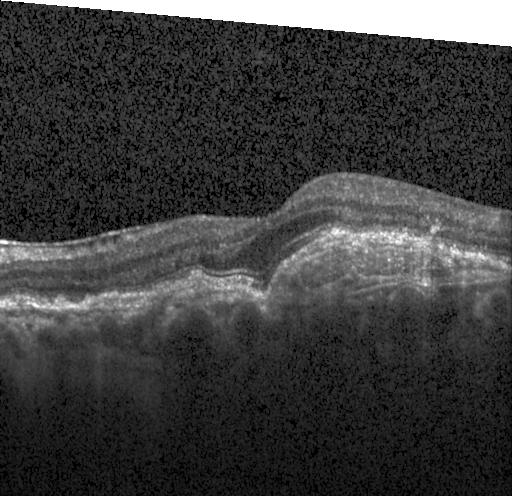

Retinal OCT B-scan · acquired on a Heidelberg Spectralis — Finding: choroidal neovascularization.